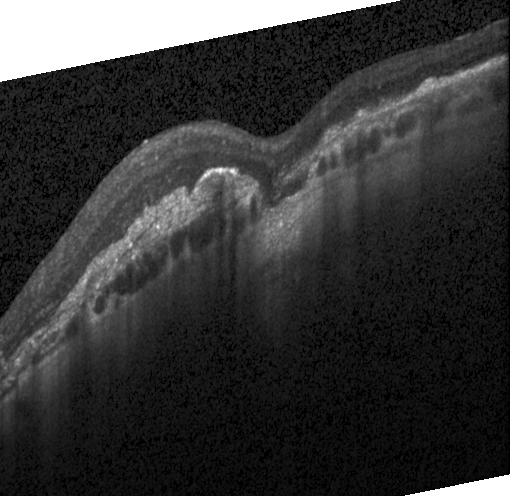 Spectral-domain OCT B-scan: choroidal neovascularization (CNV).